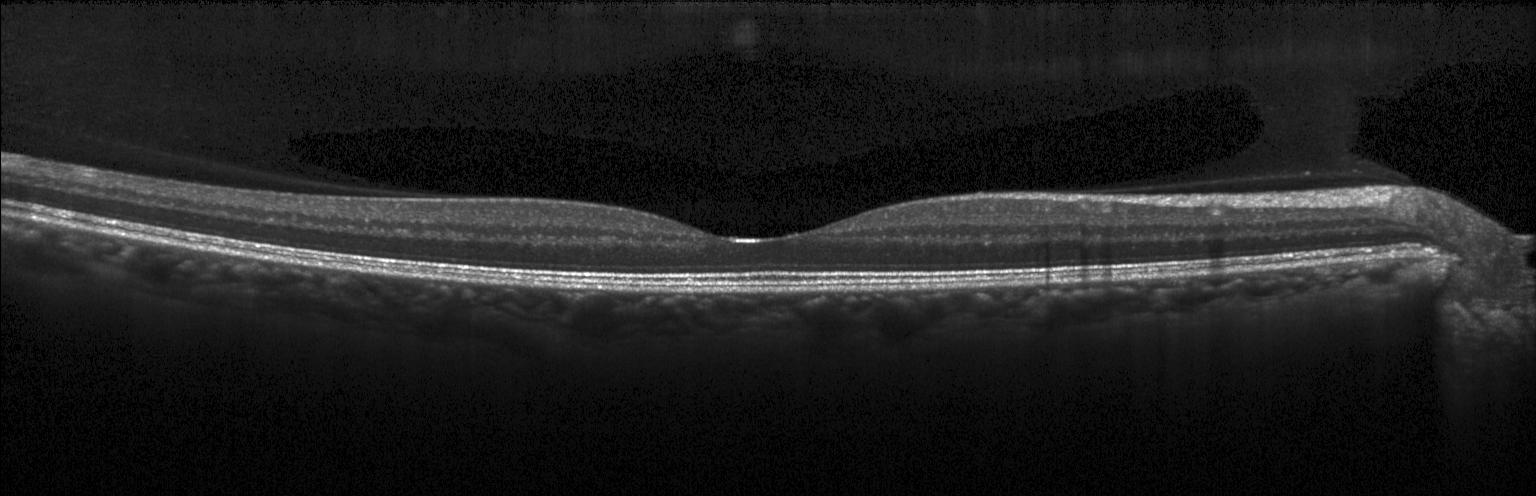

Finding: no evidence of CNV, DME, or drusen.